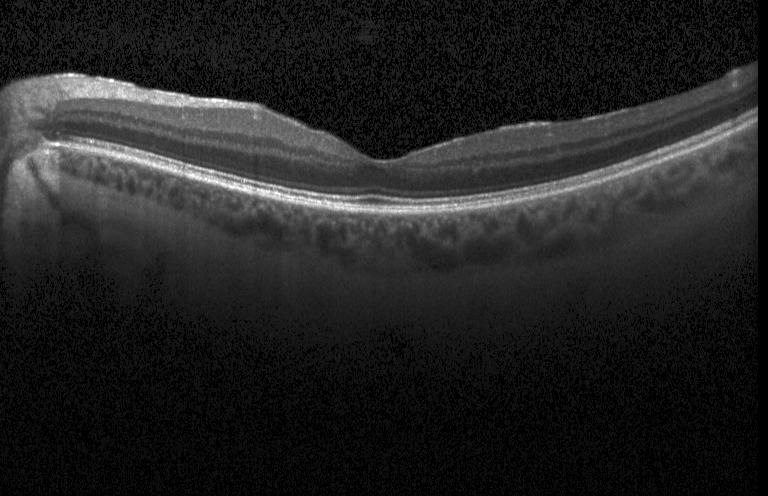
Dx: no choroidal neovascularization, diabetic macular edema, or drusen.